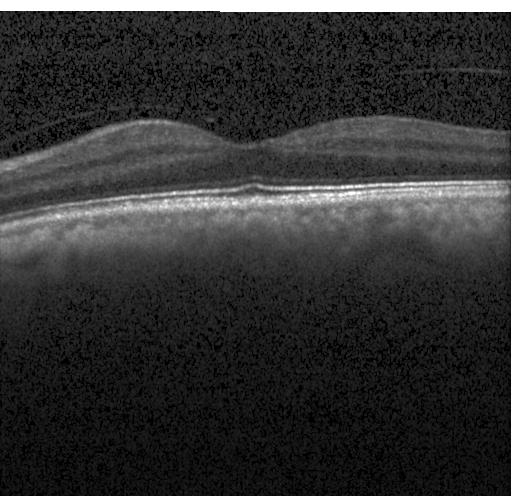 Optical coherence tomography B-scan, horizontal scan through the fovea — Assessment: no evidence of choroidal neovascularization, diabetic macular edema, or drusen.